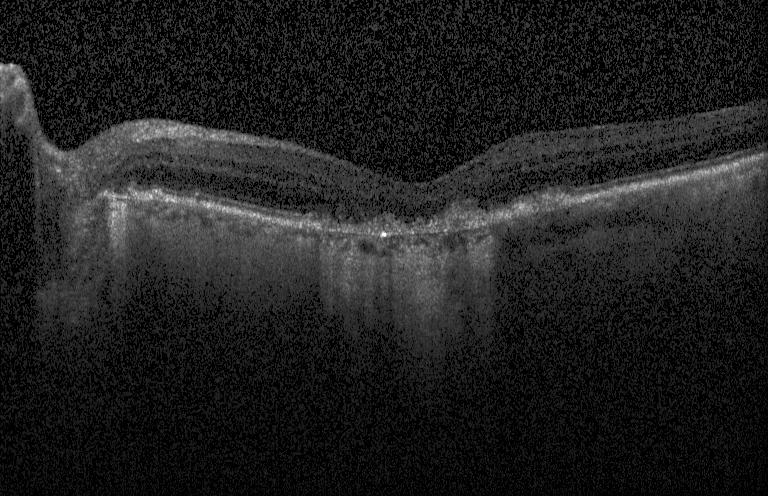

Finding: a choroidal neovascular membrane.